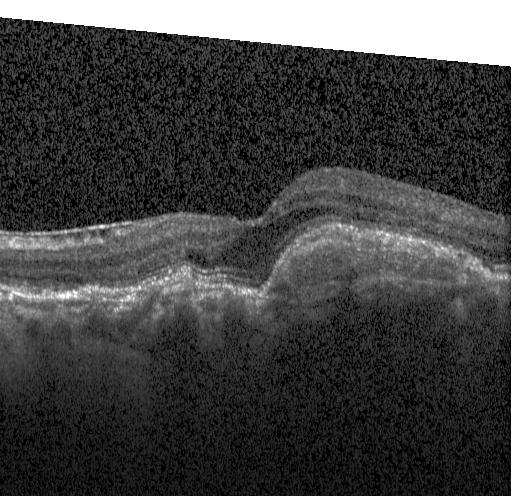 OCT B-scan — The scan shows CNV.